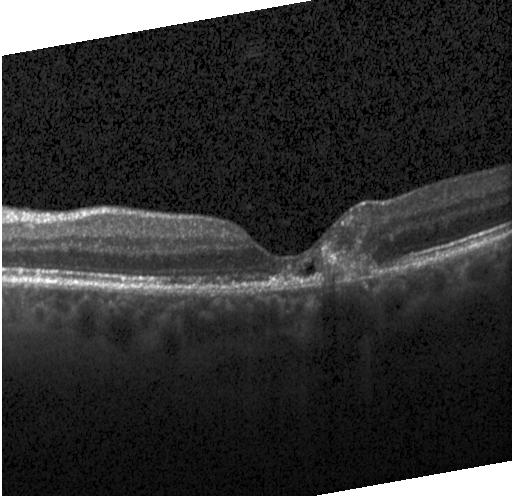 Heidelberg Spectralis OCT system, through the macula, SD-OCT, optical coherence tomography B-scan.
This B-scan demonstrates choroidal neovascularization (CNV).